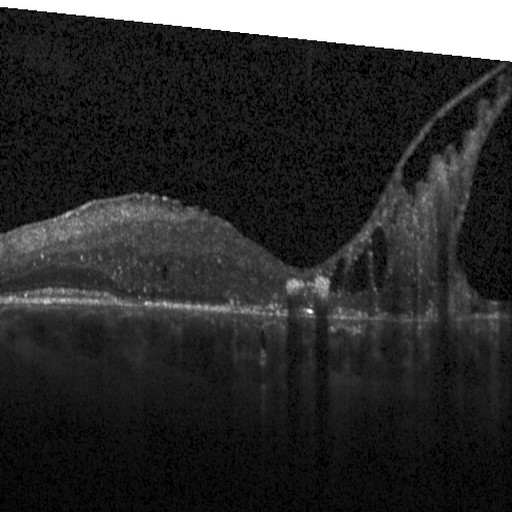
Finding: diabetic macular edema.